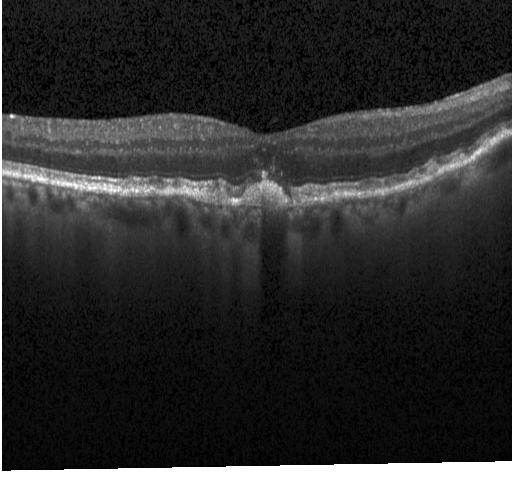
SD-OCT · OCT line scan · fovea-centered · Heidelberg Spectralis OCT system. This B-scan demonstrates multiple drusen.